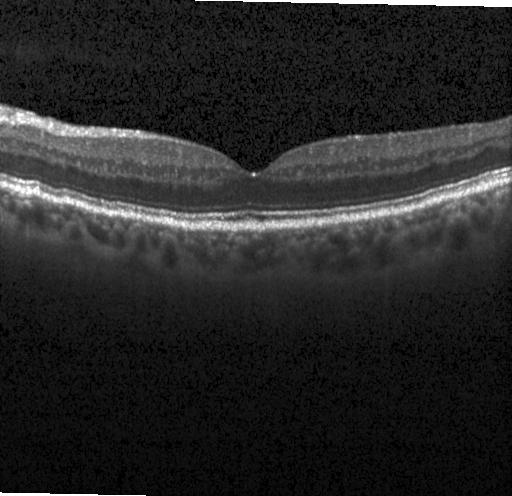 OCT finding: no evidence of CNV, DME, or drusen.